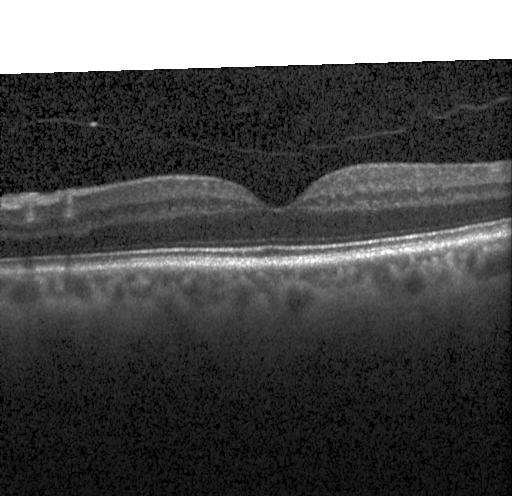 Macular scan; instrument: Heidelberg Spectralis; OCT line scan. Impression: no choroidal neovascularization, no diabetic macular edema, and no drusen.